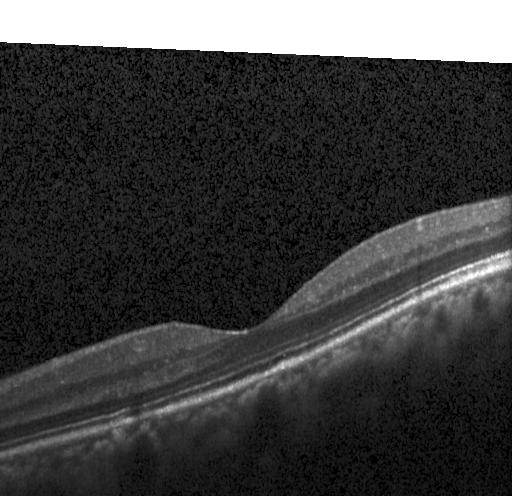 Finding: neither choroidal neovascularization, diabetic macular edema, nor drusen.